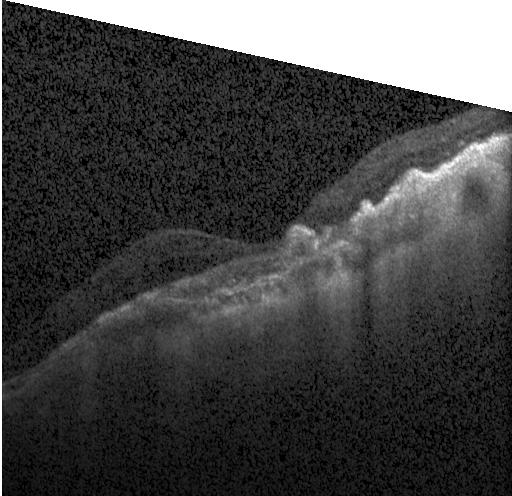 Diagnosis: a choroidal neovascular membrane.